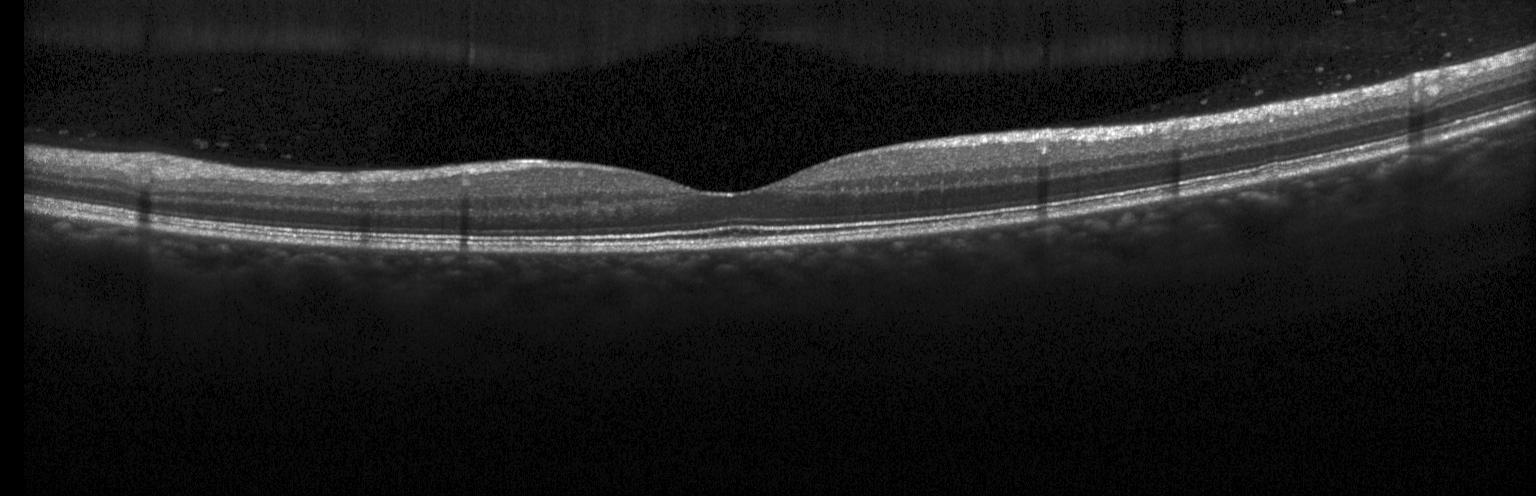
Macular OCT: neither choroidal neovascularization, diabetic macular edema, nor drusen.